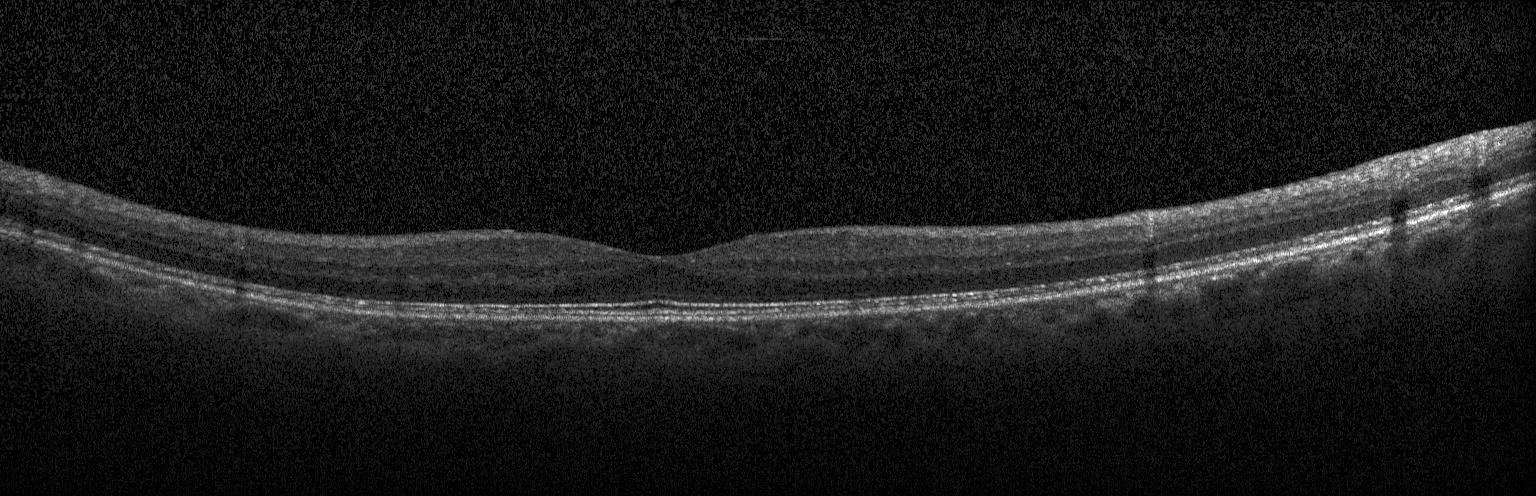

Dx: no evidence of choroidal neovascularization, diabetic macular edema, or drusen.